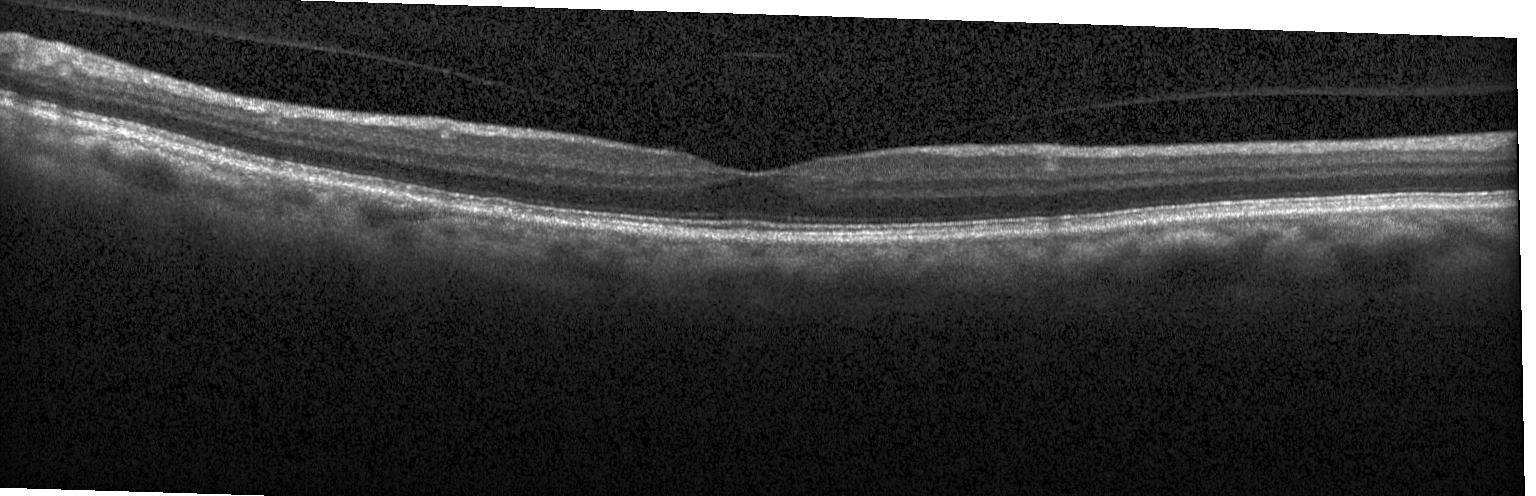 Retinal OCT cross-section showing no choroidal neovascularization, diabetic macular edema, or drusen.